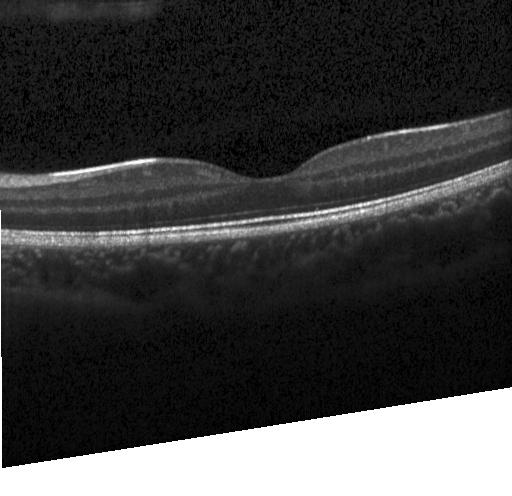
SD-OCT; optical coherence tomography scan; Heidelberg Spectralis. The scan shows no evidence of choroidal neovascularization, diabetic macular edema, or drusen.